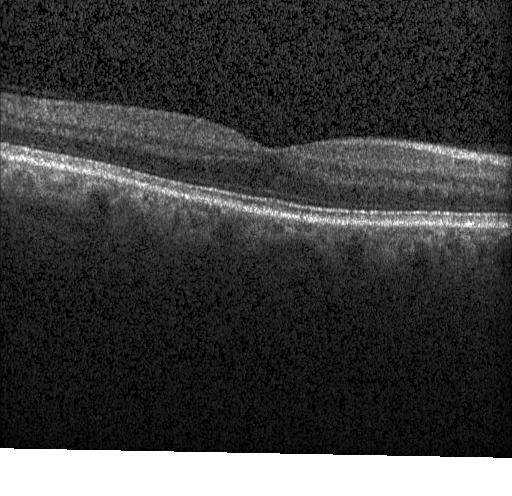 Finding: neither CNV, DME, nor drusen.